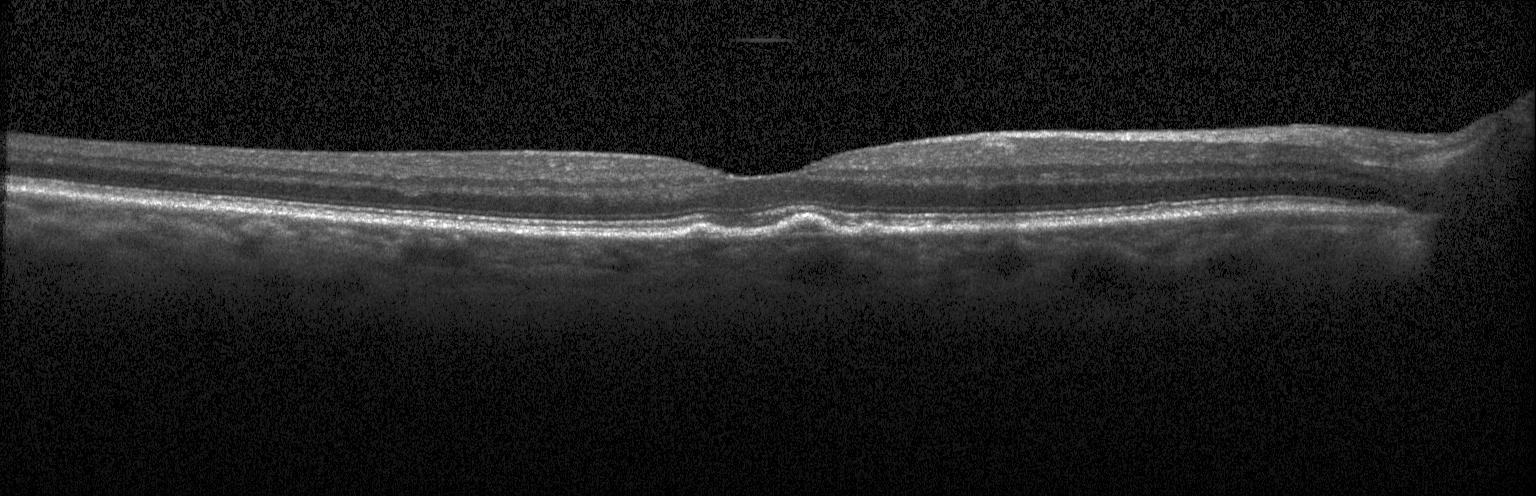 OCT B-scan
This B-scan demonstrates multiple drusen.